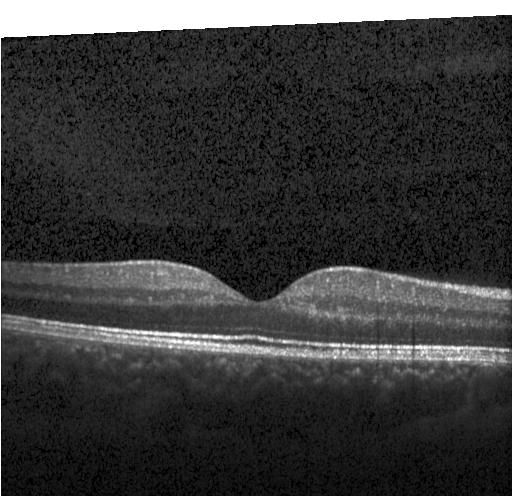

OCT B-scan showing no evidence of CNV, DME, or drusen.